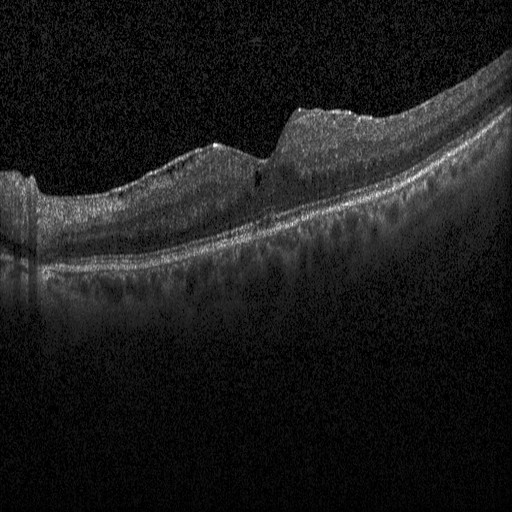

OCT B-scan showing diabetic macular edema.